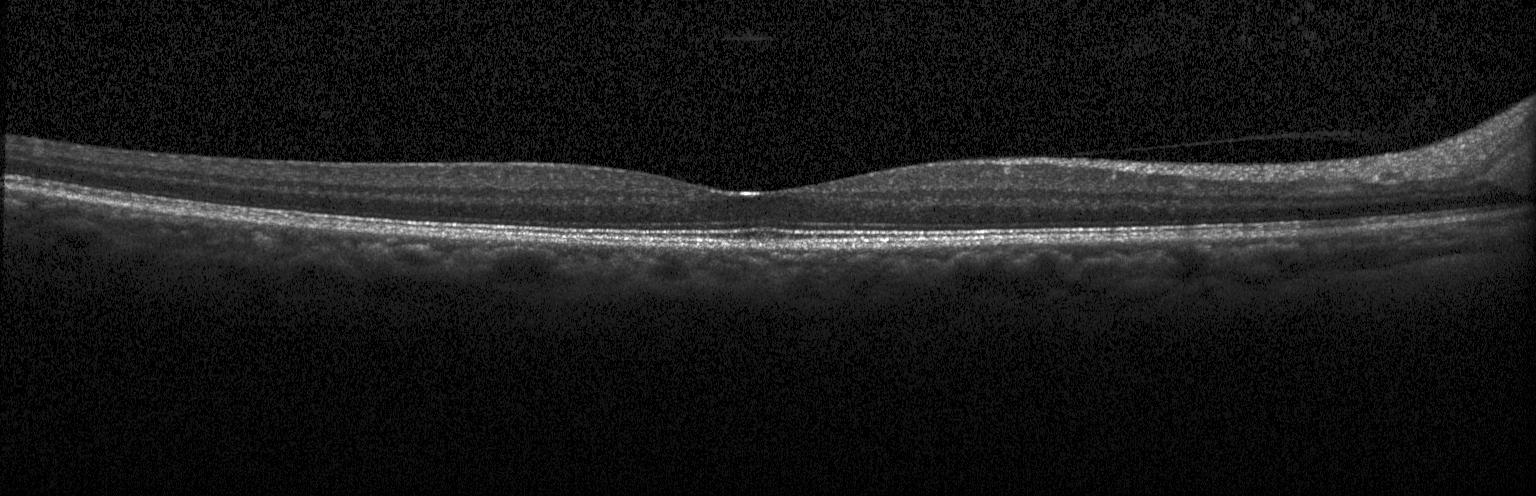 Retinal OCT cross-section. Dx: no evidence of choroidal neovascularization, diabetic macular edema, or drusen.